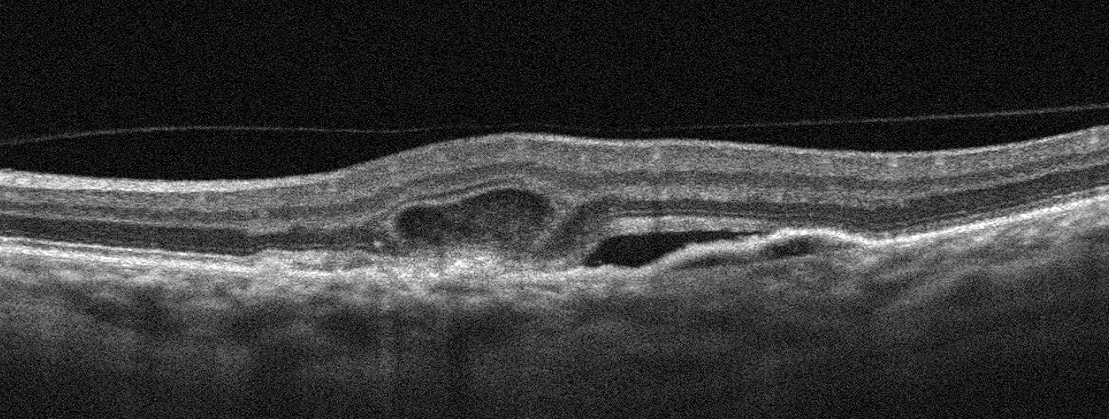
OCT B-scan showing age-related macular degeneration.